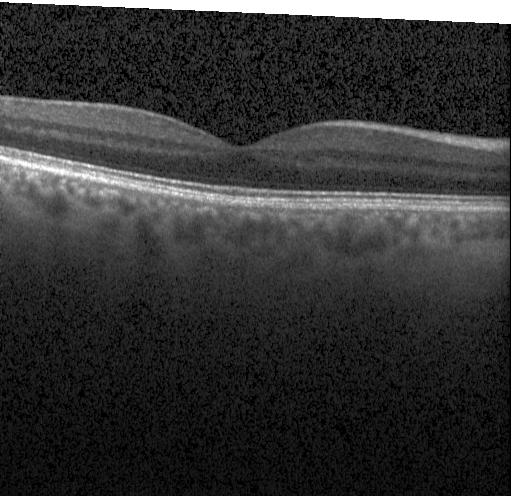

No CNV, no DME, and no drusen.